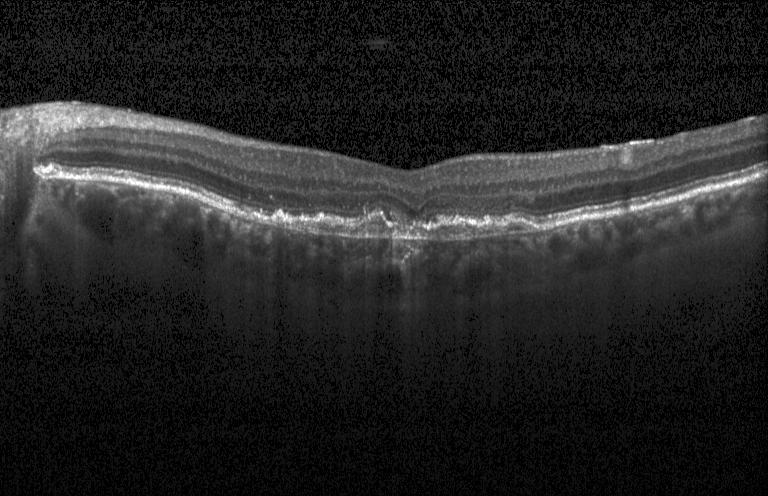

Spectral-domain OCT B-scan: CNV.